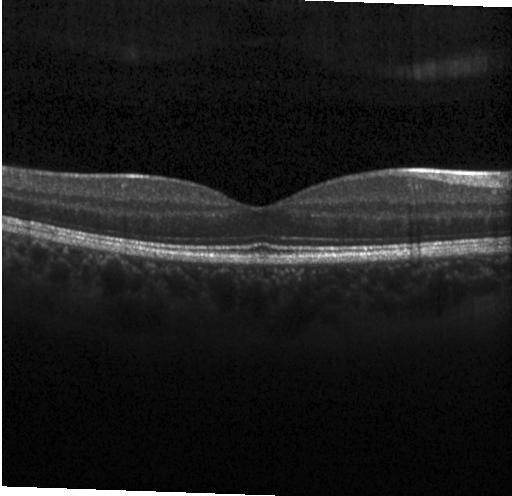

Spectral-domain optical coherence tomography, optical coherence tomography B-scan, Heidelberg Spectralis OCT system. Finding: no evidence of CNV, DME, or drusen.